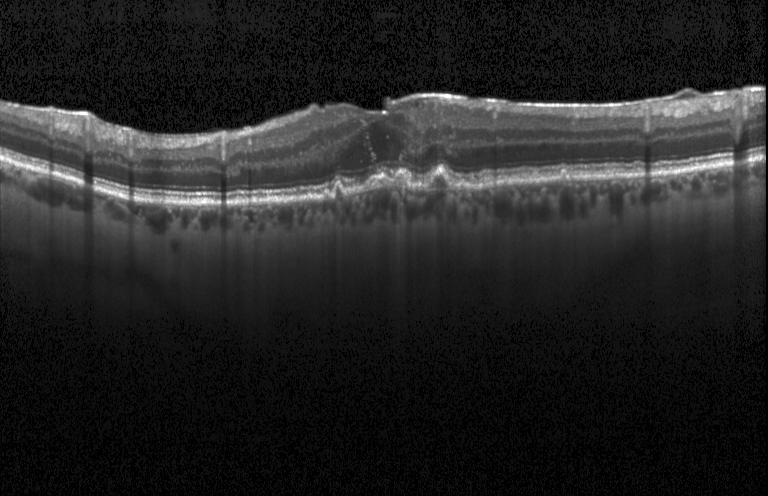

Through the macula; SD-OCT; OCT line scan
Dx: multiple drusen.